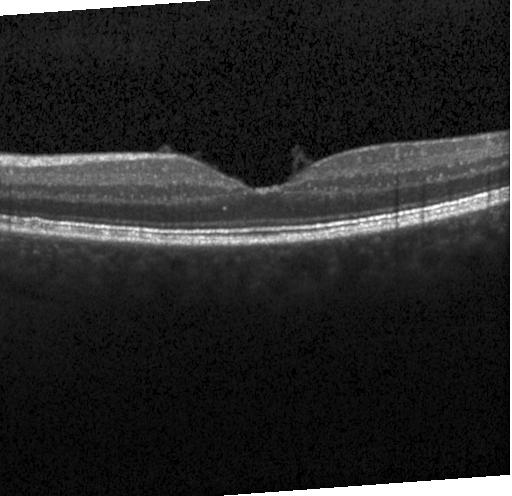

Fovea-centered, instrument: Heidelberg Spectralis, retinal OCT B-scan. This B-scan demonstrates neither CNV, DME, nor drusen.